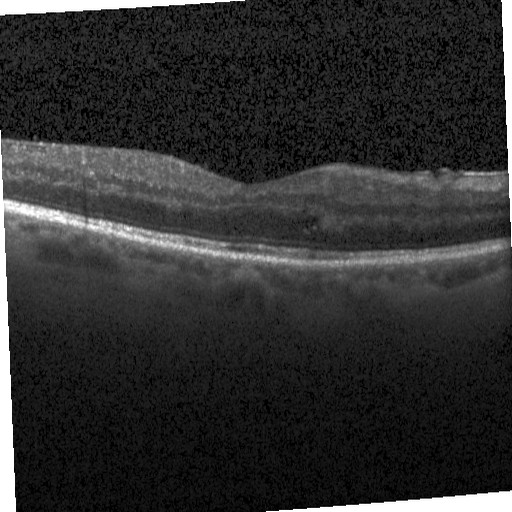
Diagnosis: diabetic macular edema (DME).